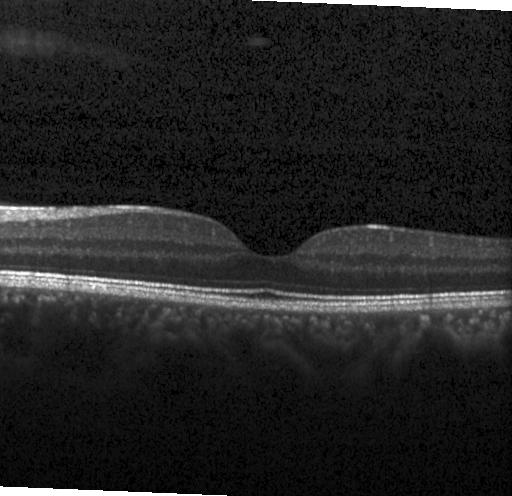

Optical coherence tomography B-scan; horizontal scan through the fovea — OCT finding: no choroidal neovascularization, no diabetic macular edema, and no drusen.